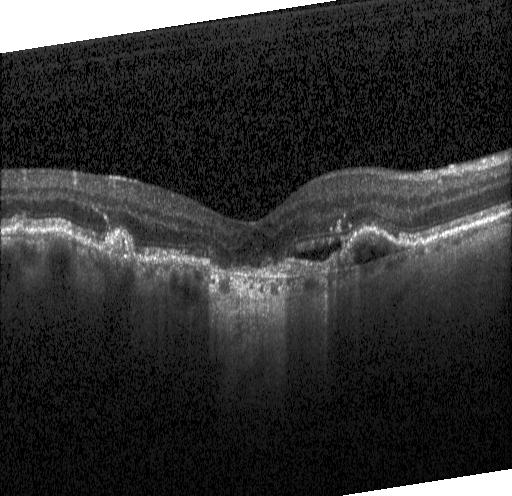
Centered on the fovea. Spectral-domain OCT. Optical coherence tomography B-scan. Heidelberg Spectralis
Assessment: a choroidal neovascular membrane.